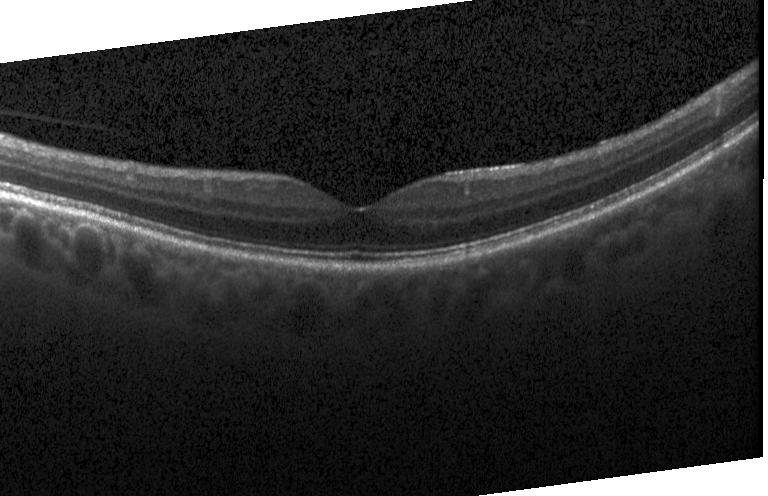
Impression: no choroidal neovascularization, no diabetic macular edema, and no drusen.